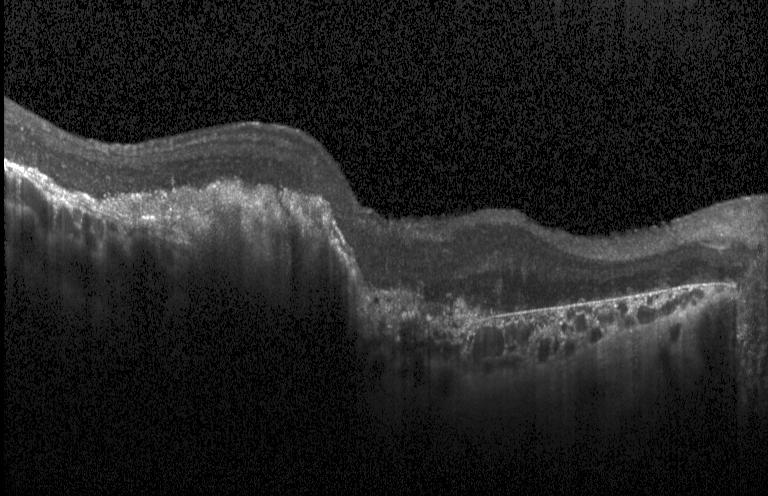
Macular OCT demonstrating a choroidal neovascular membrane.